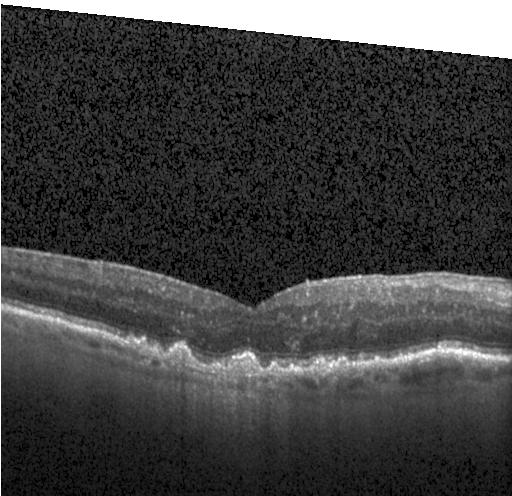
A choroidal neovascular membrane.